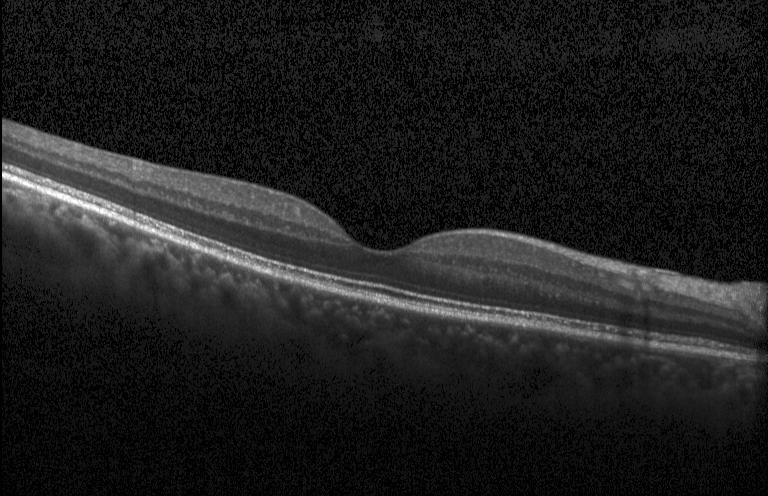
Spectral-domain OCT; optical coherence tomography B-scan; through the macula; acquired on a Heidelberg Spectralis — Diagnosis: no CNV, no DME, and no drusen.